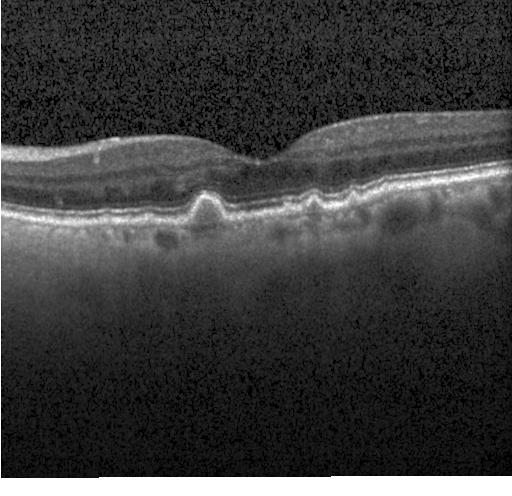
OCT B-scan showing drusen.